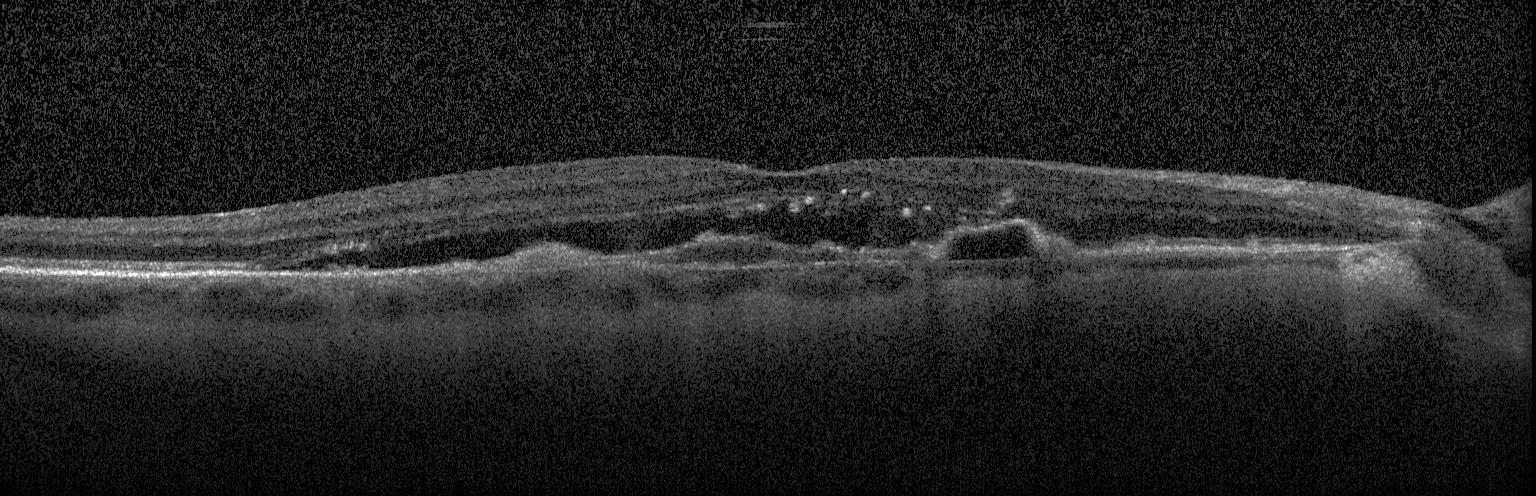
Spectral-domain optical coherence tomography; Heidelberg Spectralis OCT system; retinal OCT B-scan.
The scan shows choroidal neovascularization (CNV).